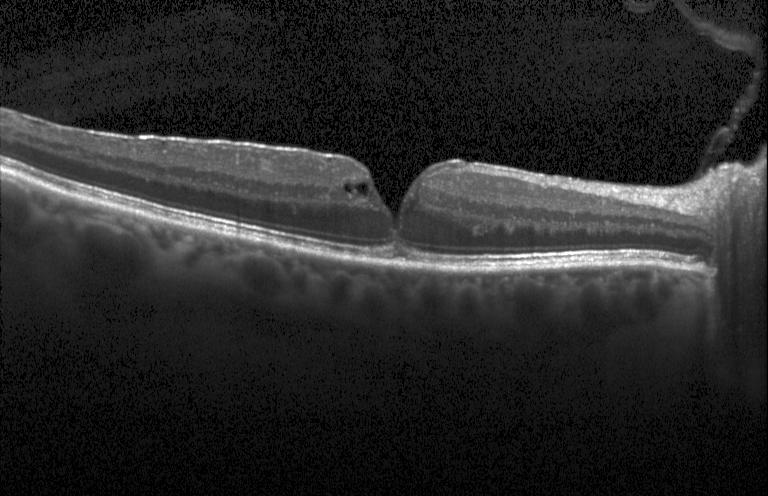 Macular OCT demonstrating DME.